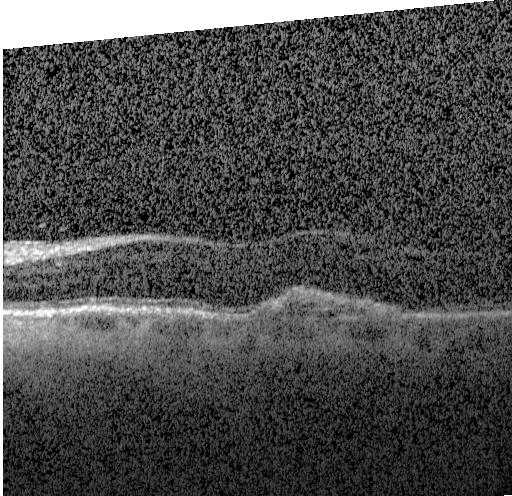

Impression: choroidal neovascularization.